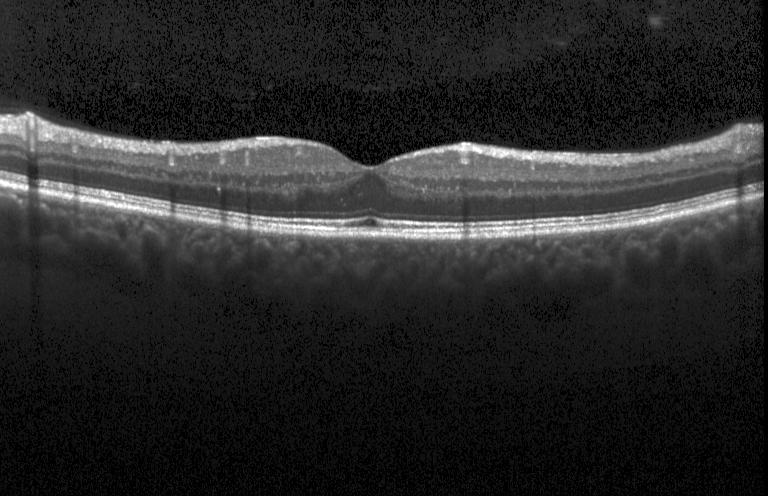
OCT B-scan showing no evidence of choroidal neovascularization, diabetic macular edema, or drusen.